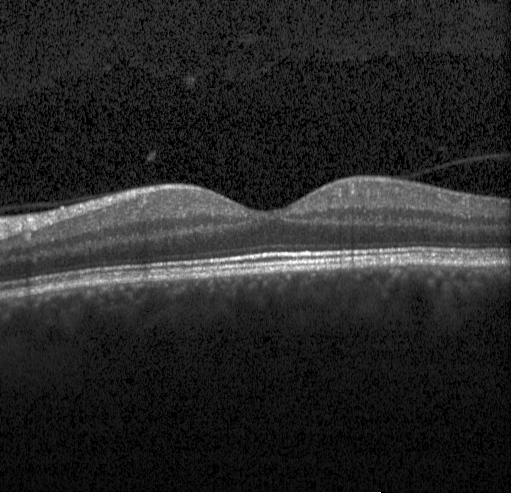

OCT B-scan.
Dx: no CNV, DME, or drusen.